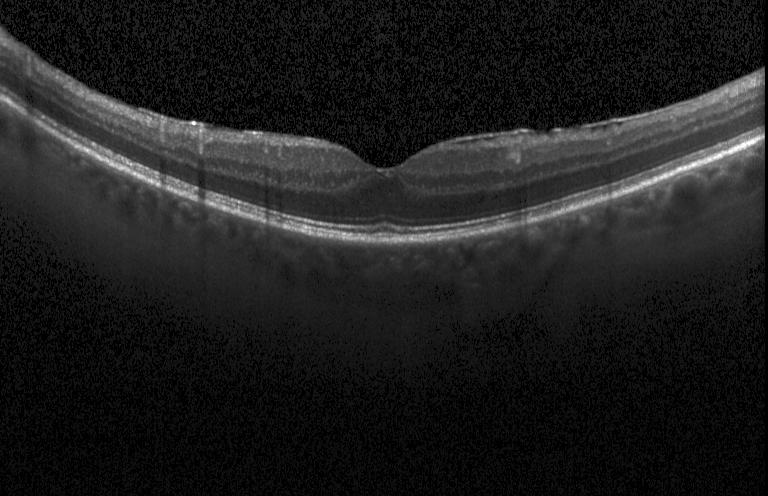 Retinal OCT cross-section.
Neither choroidal neovascularization, diabetic macular edema, nor drusen.